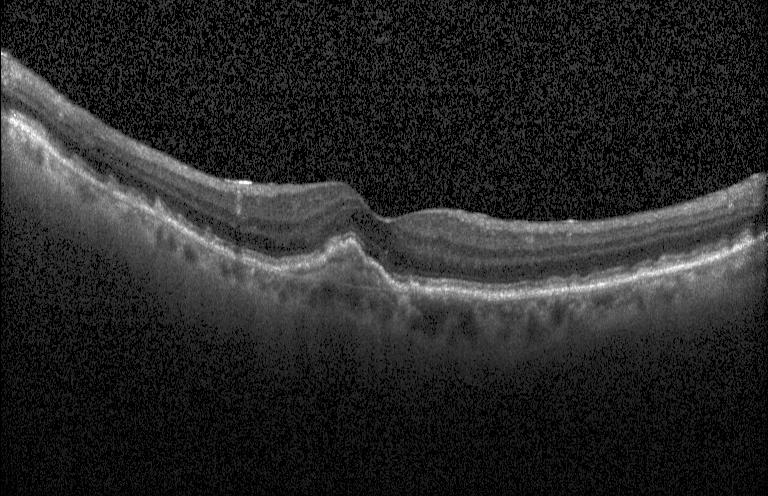
This B-scan demonstrates choroidal neovascularization.